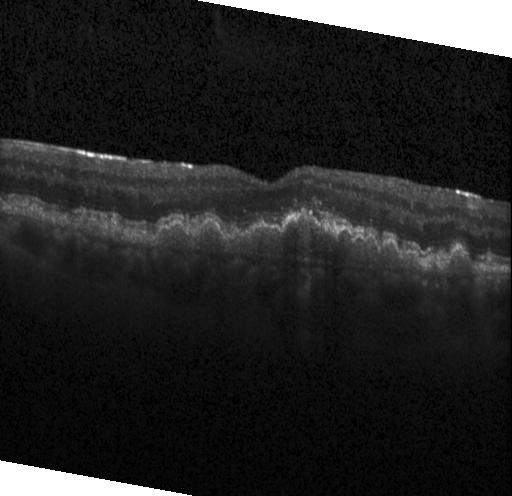
Spectral-domain optical coherence tomography; instrument: Heidelberg Spectralis; OCT B-scan — A choroidal neovascular membrane.